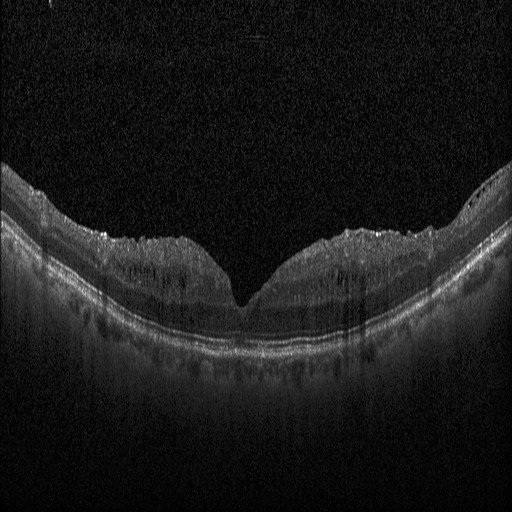
Heidelberg Spectralis OCT system; fovea-centered; optical coherence tomography scan; spectral-domain OCT.
Diagnosis: diabetic macular edema.